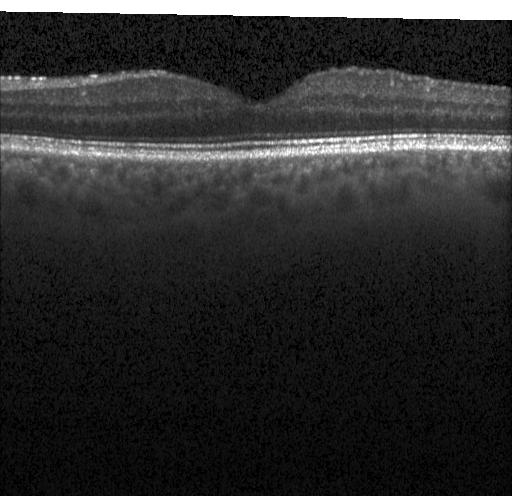 OCT finding: no choroidal neovascularization, no diabetic macular edema, and no drusen.